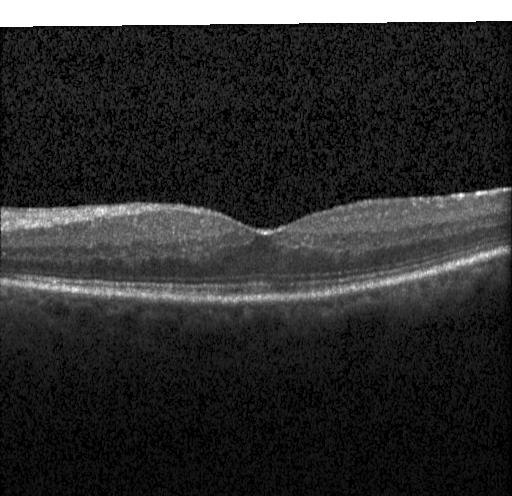

Retinal OCT B-scan. This B-scan demonstrates no choroidal neovascularization, no diabetic macular edema, and no drusen.